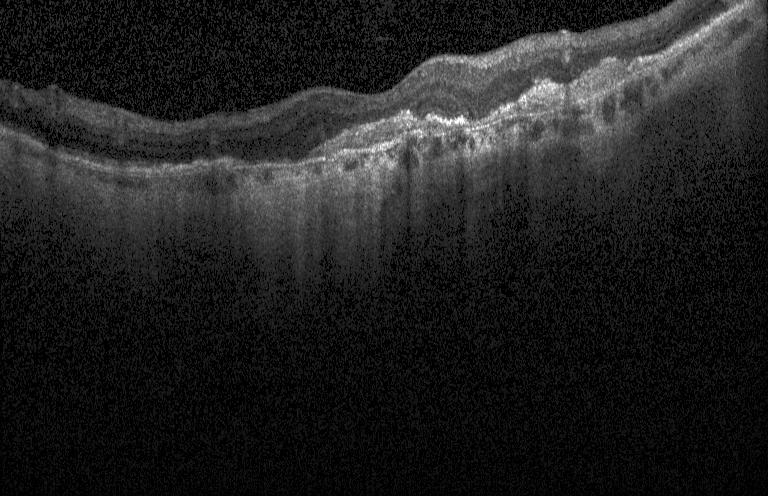

OCT B-scan; SD-OCT.
Assessment: CNV.